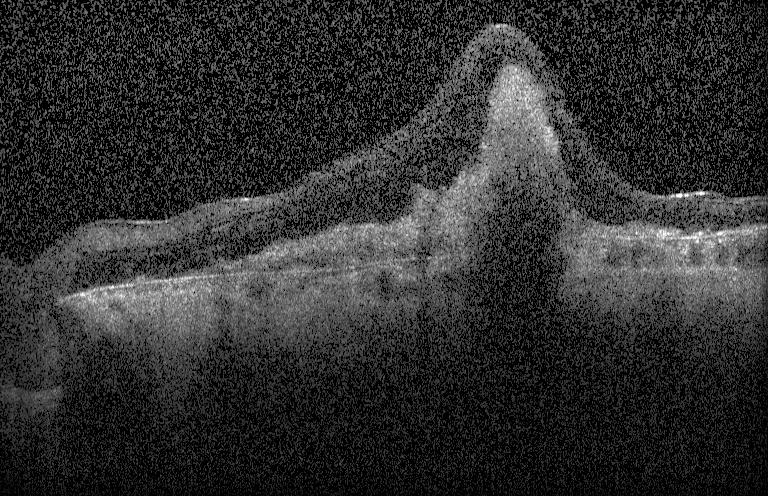 Spectral-domain OCT · optical coherence tomography B-scan · acquired on a Heidelberg Spectralis · horizontal scan through the fovea. Diagnosis: choroidal neovascularization (CNV).